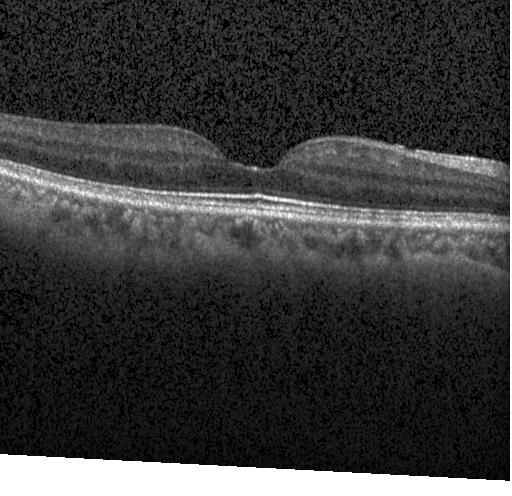 Diagnosis: no evidence of choroidal neovascularization, diabetic macular edema, or drusen.